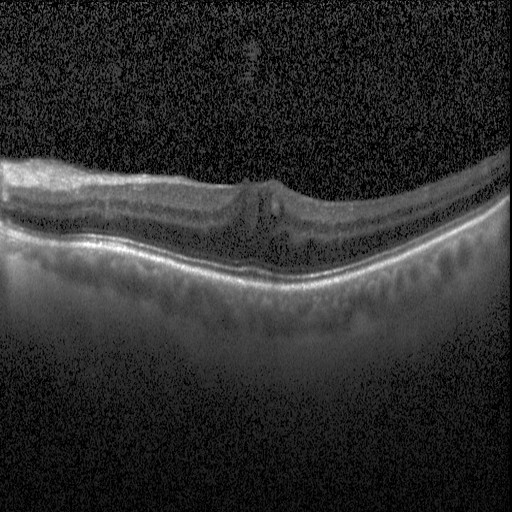 Diabetic macular edema (DME).